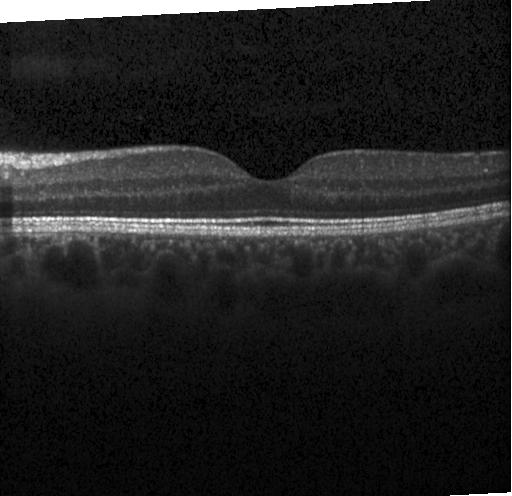
Optical coherence tomography B-scan.
Impression: neither choroidal neovascularization, diabetic macular edema, nor drusen.